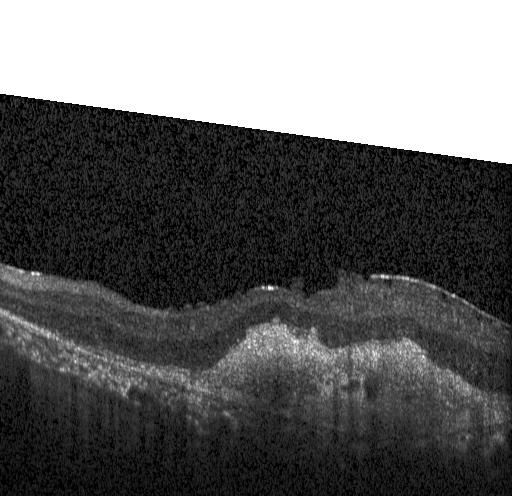
OCT line scan; acquired on a Heidelberg Spectralis; horizontal scan through the fovea. OCT finding: a choroidal neovascular membrane.